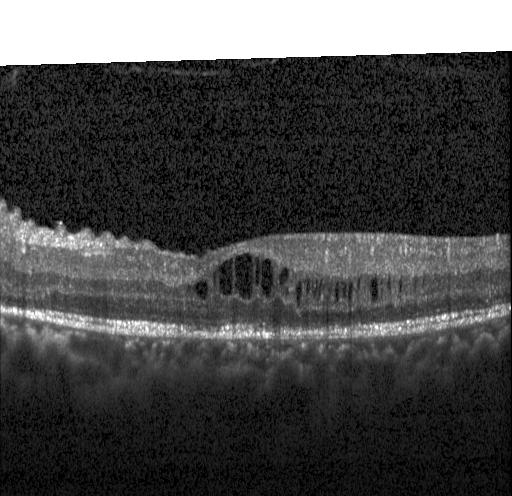 Impression: DME.